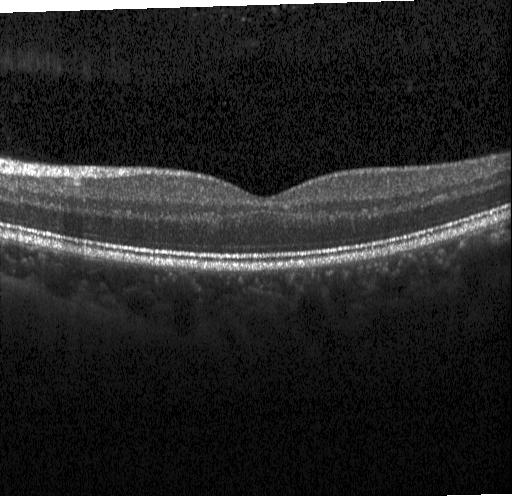

OCT B-scan showing no choroidal neovascularization, no diabetic macular edema, and no drusen.